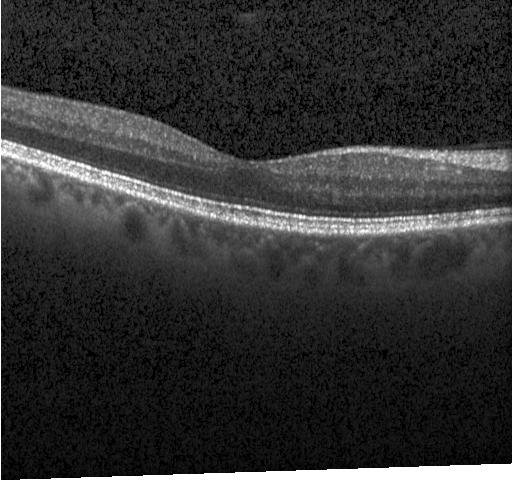

Heidelberg Spectralis. Retinal OCT cross-section. Fovea-centered. Spectral-domain OCT — Assessment: no evidence of CNV, DME, or drusen.